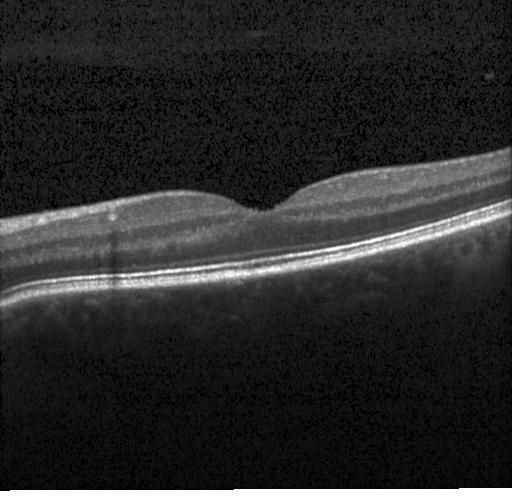

Diagnosis: no CNV, no DME, and no drusen.